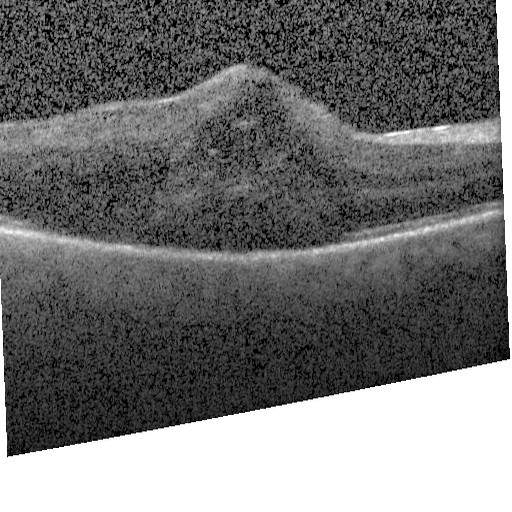
Optical coherence tomography scan. Fovea-centered. SD-OCT
Finding: diabetic macular edema (DME).